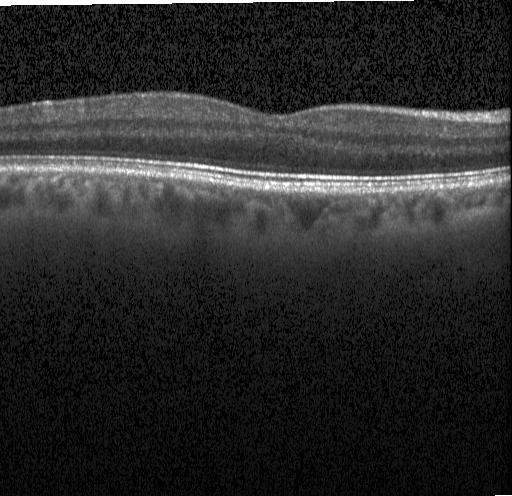 Retinal OCT cross-section. Finding: no evidence of choroidal neovascularization, diabetic macular edema, or drusen.